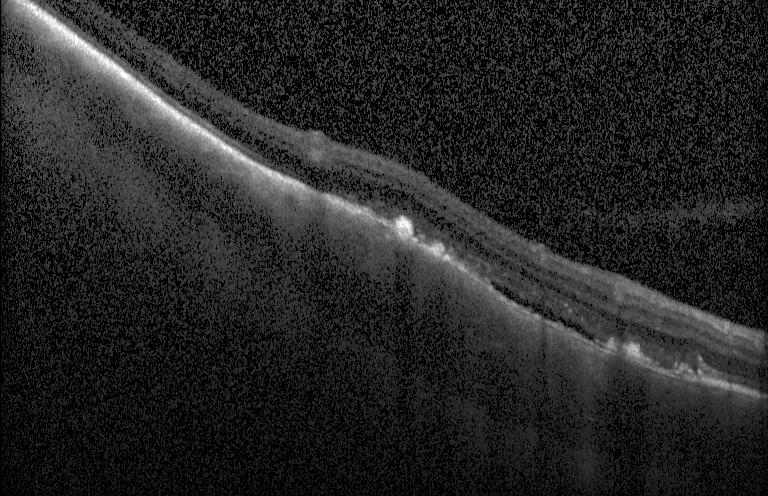

Heidelberg Spectralis OCT system; optical coherence tomography scan; centered on the fovea; SD-OCT.
Dx: a choroidal neovascular membrane.